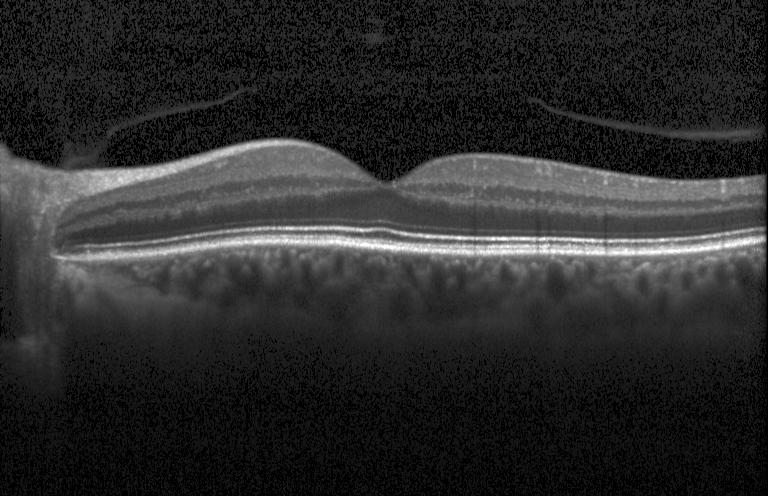 Impression: no evidence of choroidal neovascularization, diabetic macular edema, or drusen.